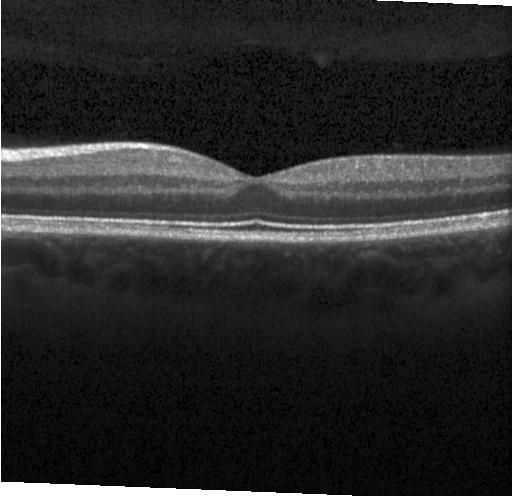 Retinal OCT B-scan. Macular scan. SD-OCT.
Impression: no CNV, no DME, and no drusen.